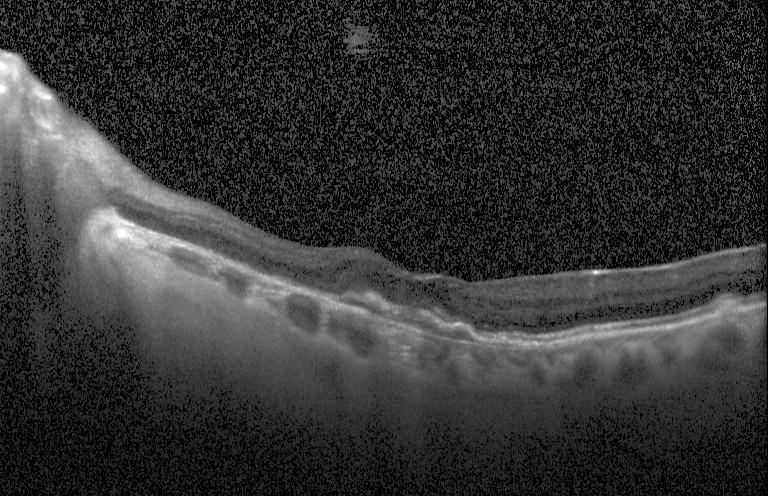

Optical coherence tomography B-scan; horizontal scan through the fovea; acquired on a Heidelberg Spectralis — Diagnosis: CNV.